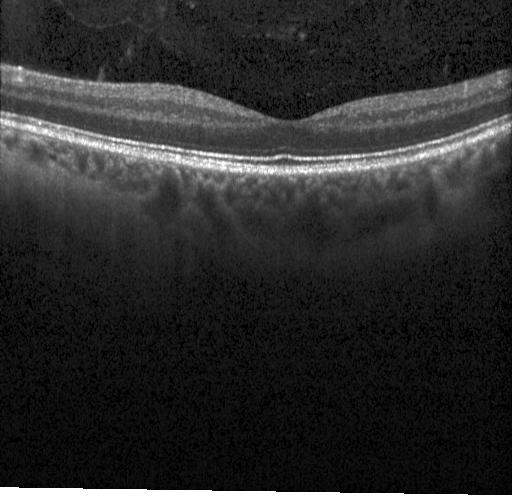
OCT line scan. Spectral-domain optical coherence tomography. Impression: no choroidal neovascularization, no diabetic macular edema, and no drusen.